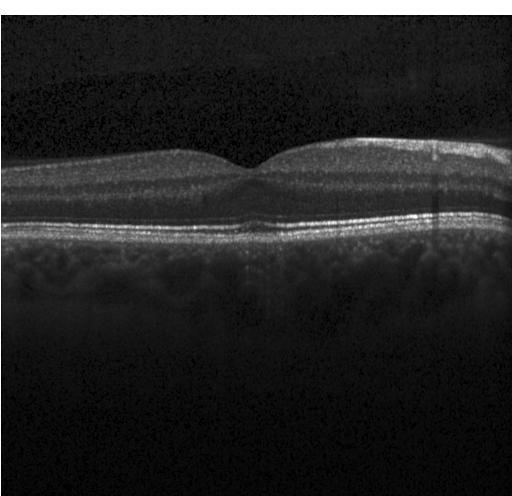

Spectral-domain OCT; through the macula; acquired on a Heidelberg Spectralis; optical coherence tomography scan — Finding: no choroidal neovascularization, no diabetic macular edema, and no drusen.